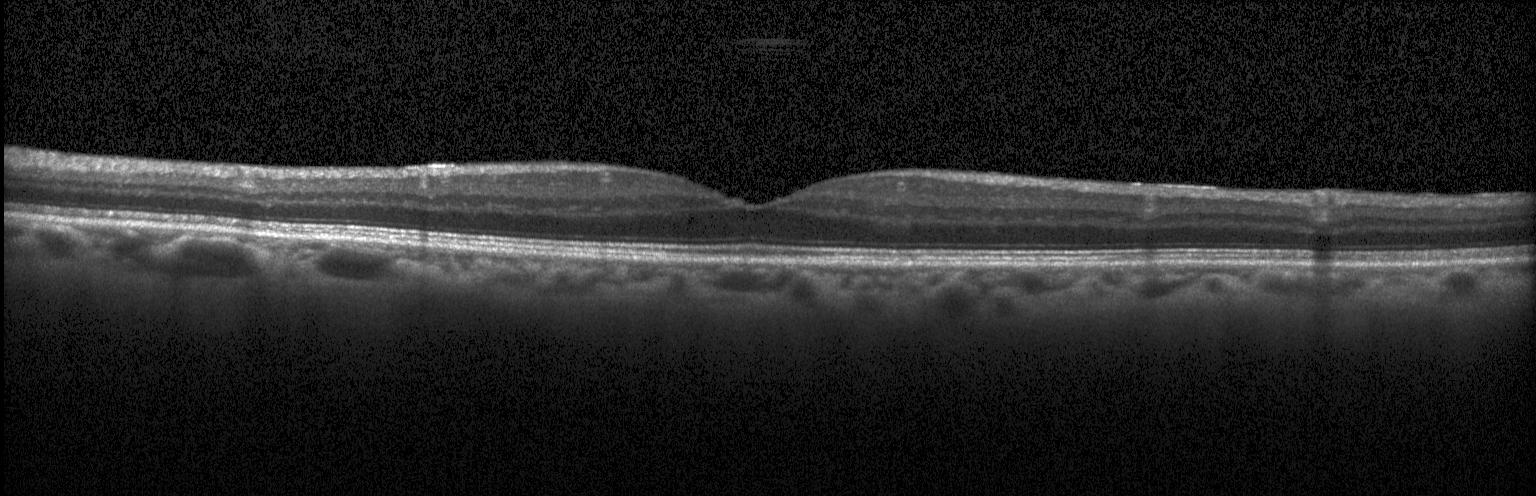
Impression: neither CNV, DME, nor drusen.